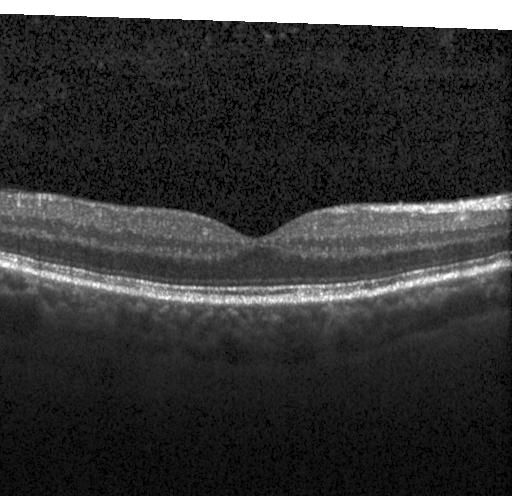
Heidelberg Spectralis OCT system, OCT B-scan — Impression: no evidence of choroidal neovascularization, diabetic macular edema, or drusen.